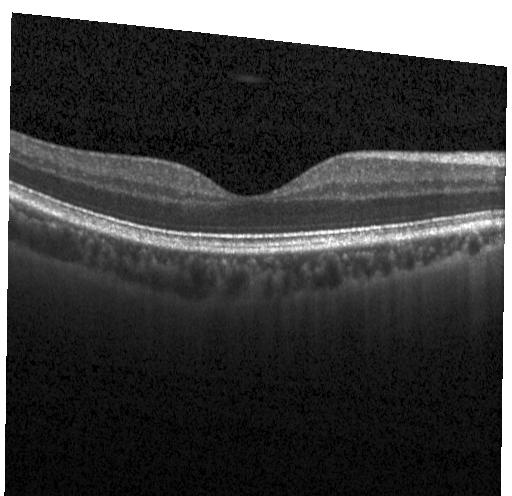

Optical coherence tomography scan — Macular OCT: neither choroidal neovascularization, diabetic macular edema, nor drusen.